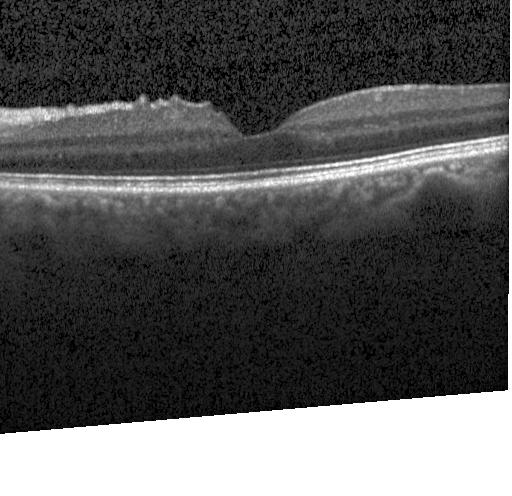

OCT B-scan — Impression: no choroidal neovascularization, diabetic macular edema, or drusen.